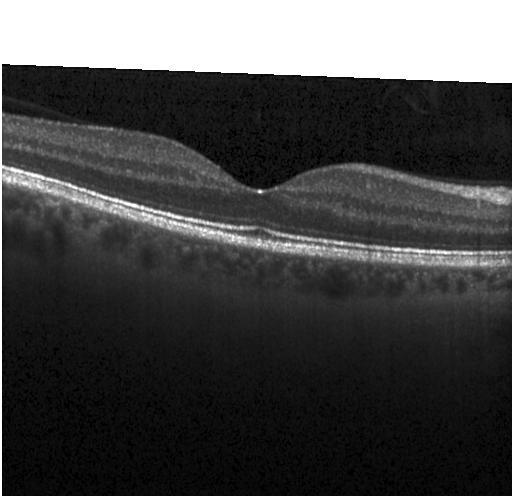

The scan shows no choroidal neovascularization, diabetic macular edema, or drusen.